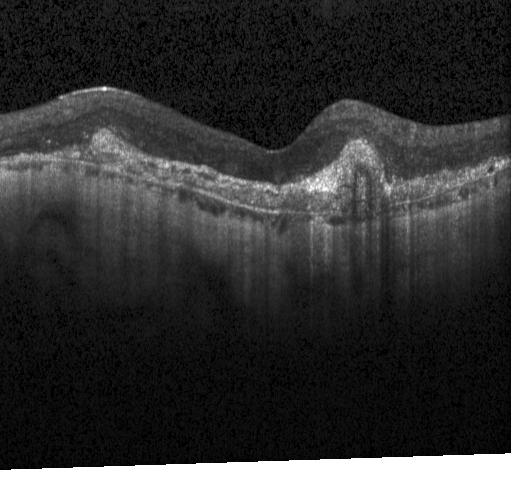

Spectral-domain OCT · OCT B-scan · Heidelberg Spectralis.
Macular OCT: a choroidal neovascular membrane.